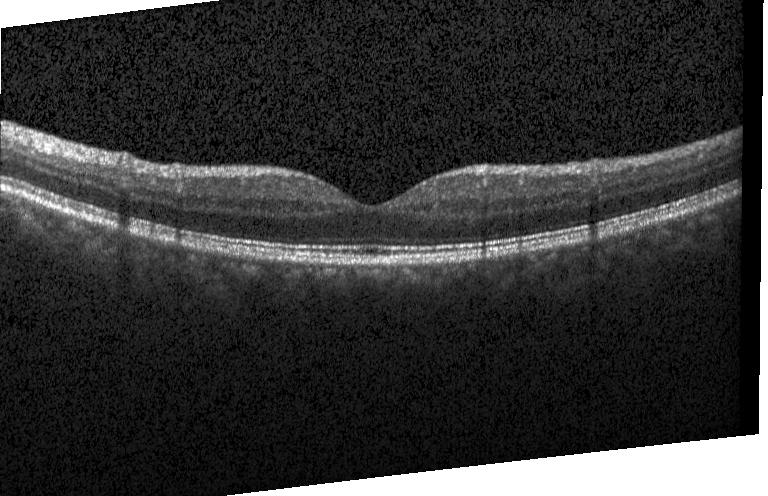

This B-scan demonstrates no evidence of choroidal neovascularization, diabetic macular edema, or drusen.